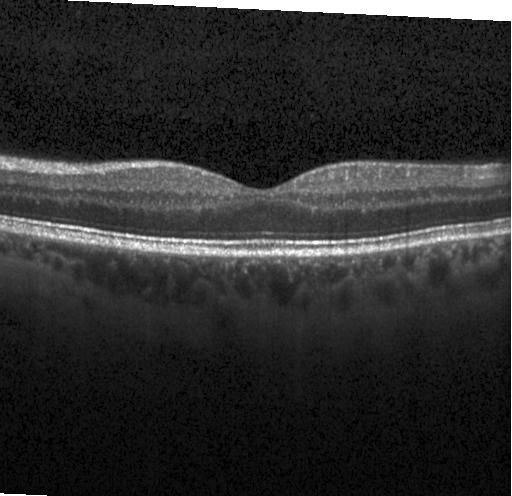

Diagnosis: neither choroidal neovascularization, diabetic macular edema, nor drusen.